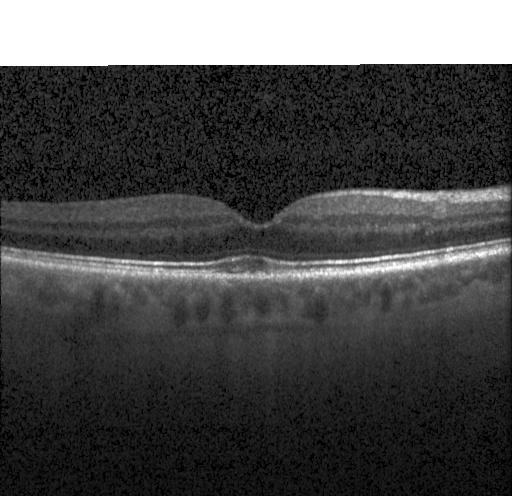

Heidelberg Spectralis OCT system, centered on the fovea, spectral-domain optical coherence tomography, optical coherence tomography scan — Diagnosis: no choroidal neovascularization, no diabetic macular edema, and no drusen.